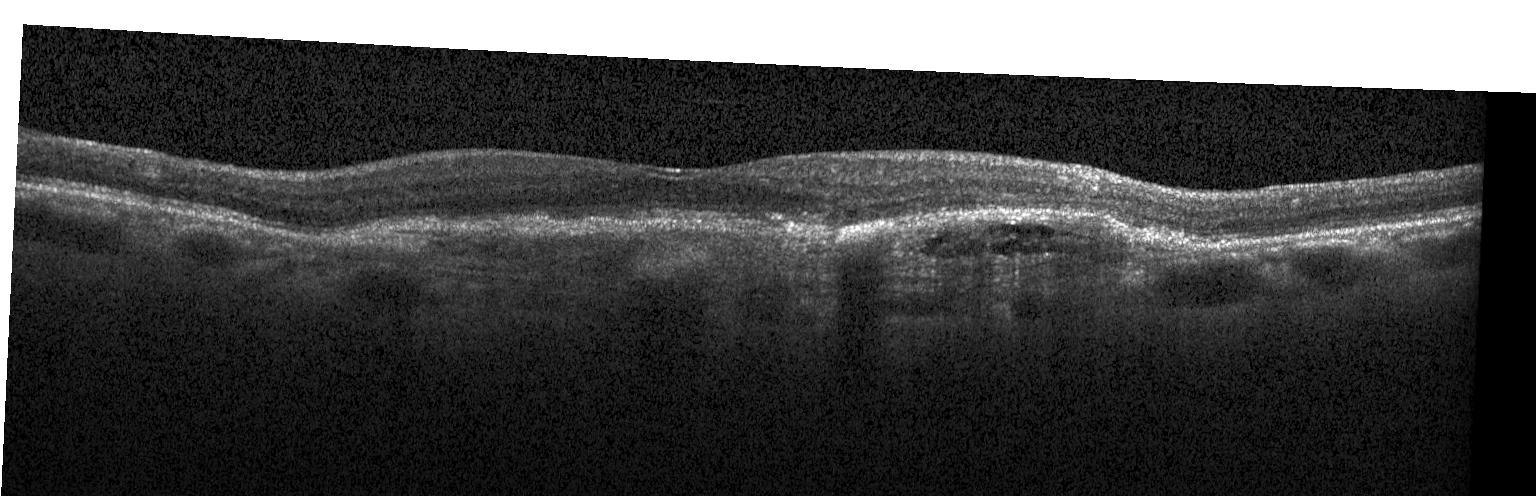 OCT B-scan, horizontal scan through the fovea
Finding: a choroidal neovascular membrane.